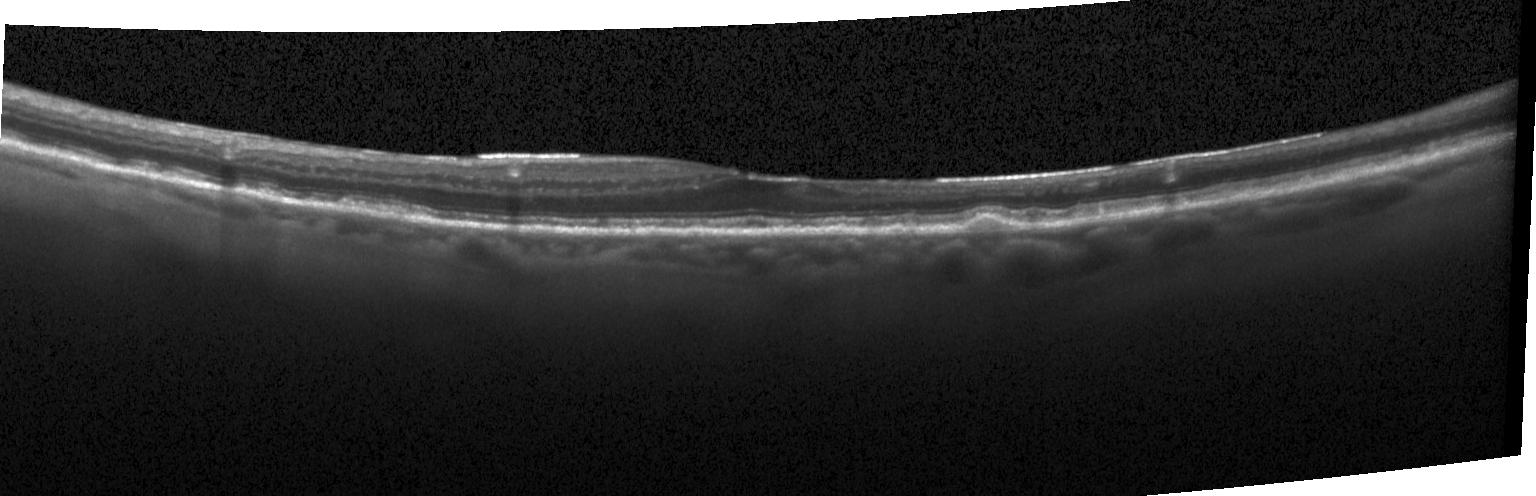

Fovea-centered, instrument: Heidelberg Spectralis, retinal OCT B-scan
The scan shows multiple drusen.